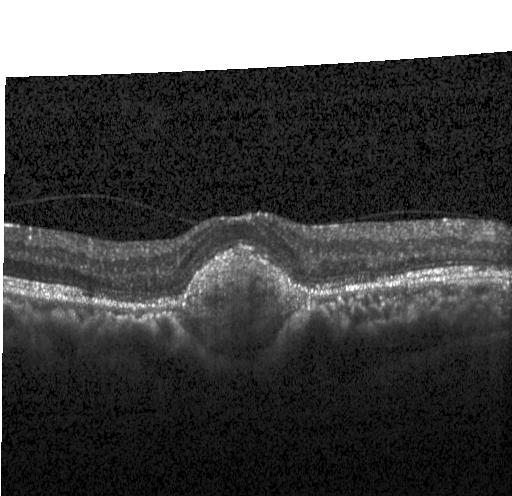

Diagnosis: CNV.